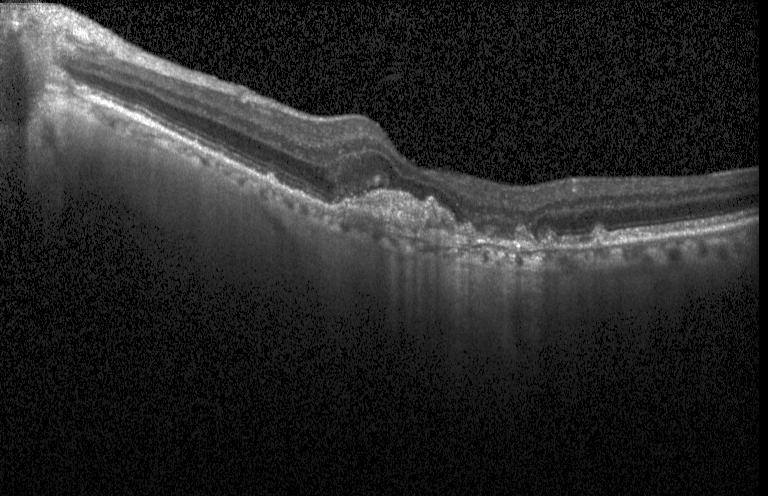

Retinal OCT cross-section showing a choroidal neovascular membrane.